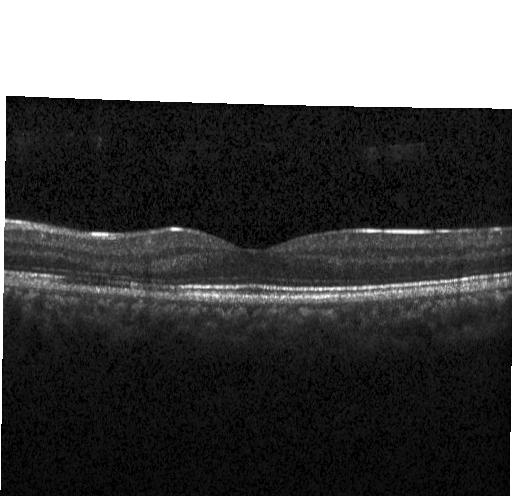 Optical coherence tomography B-scan. Diagnosis: no CNV, DME, or drusen.